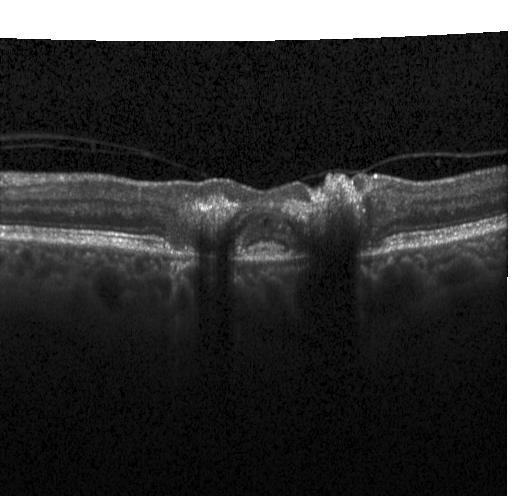
Finding: choroidal neovascularization.